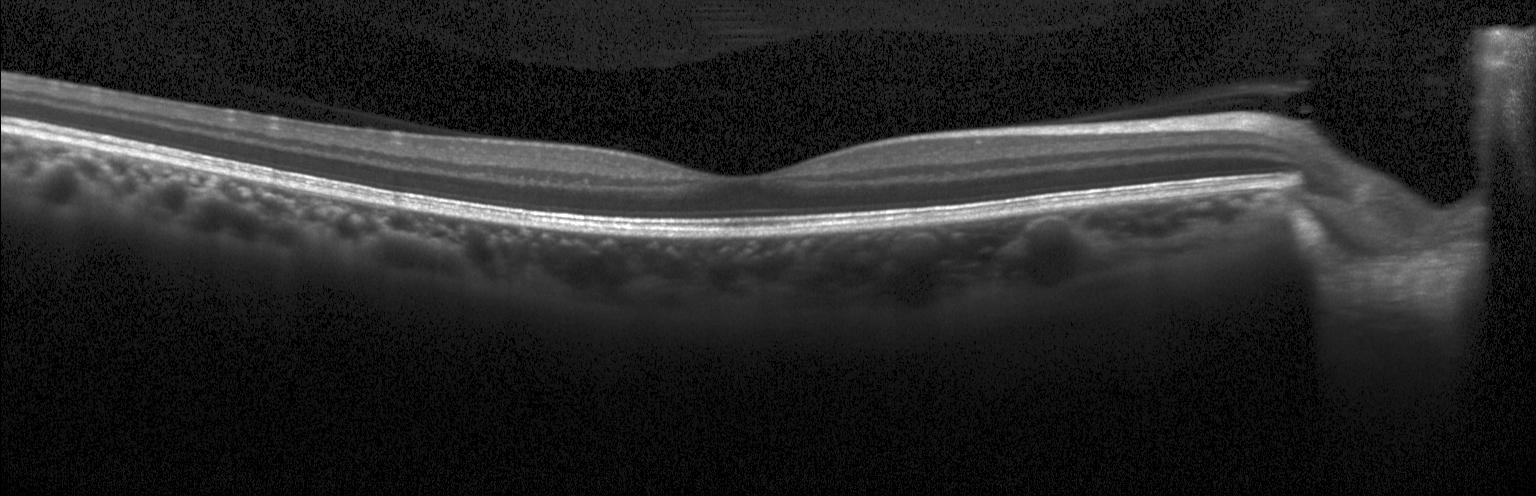
Optical coherence tomography scan.
No choroidal neovascularization, diabetic macular edema, or drusen.